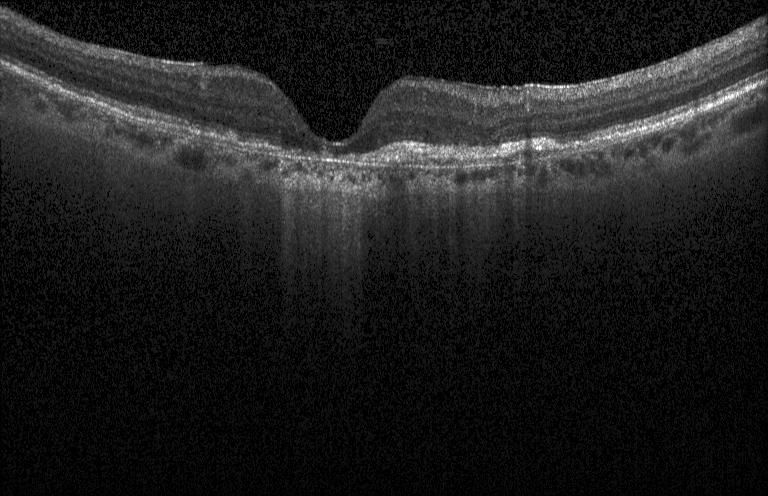
Finding: a choroidal neovascular membrane.